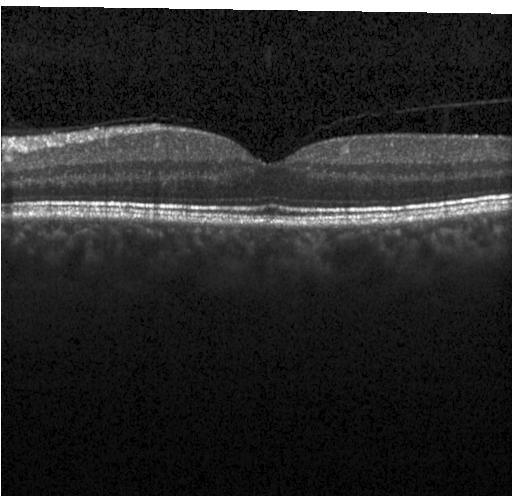

Through the macula, instrument: Heidelberg Spectralis, OCT B-scan.
Finding: no choroidal neovascularization, diabetic macular edema, or drusen.